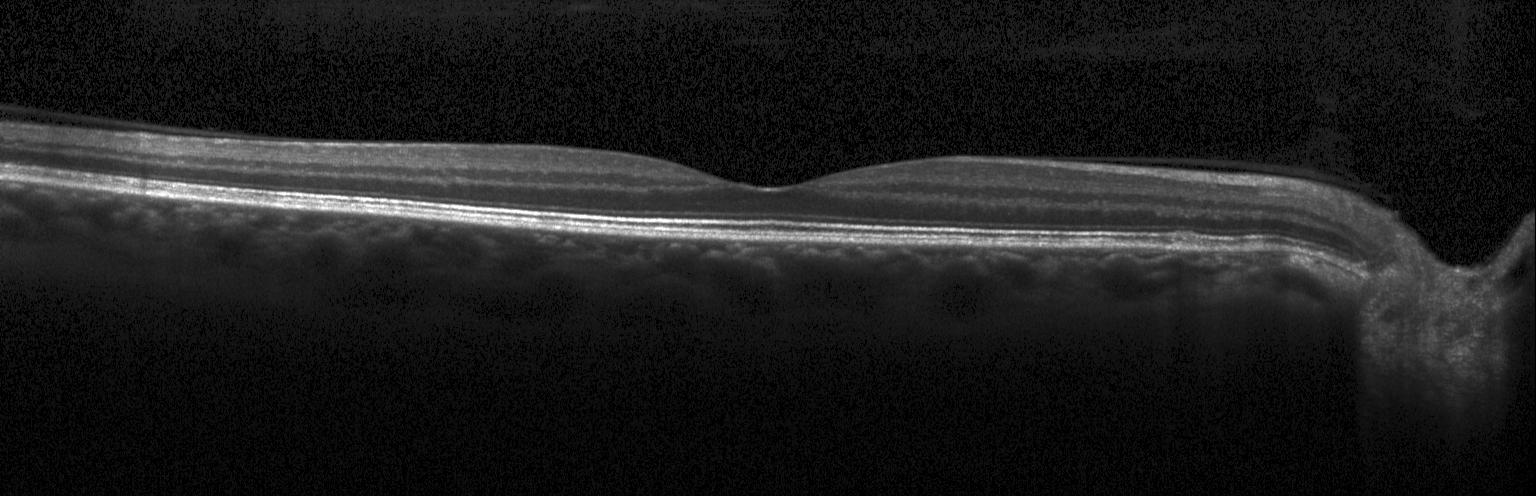

Retinal OCT cross-section
Finding: no evidence of choroidal neovascularization, diabetic macular edema, or drusen.